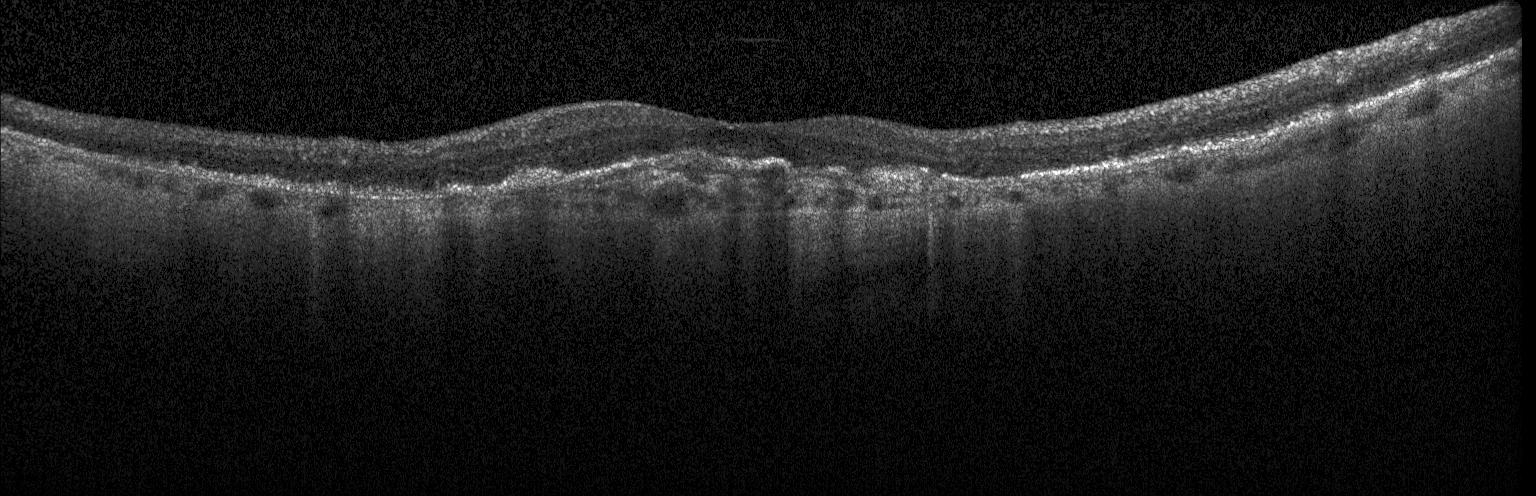
Dx: a choroidal neovascular membrane.